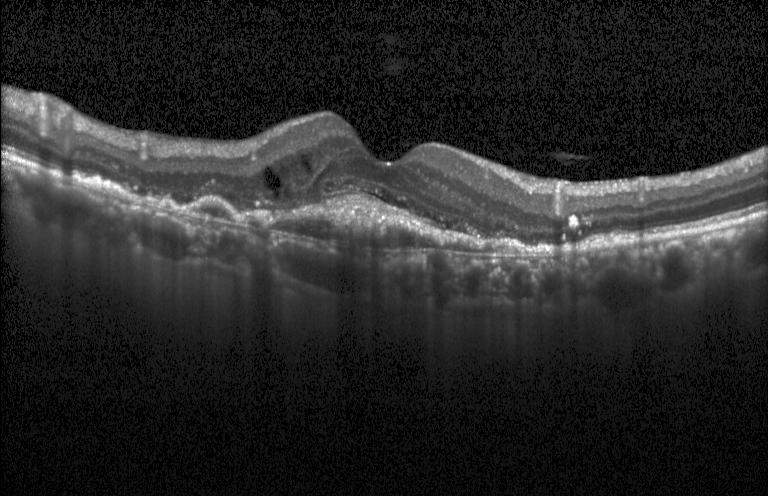
CNV.